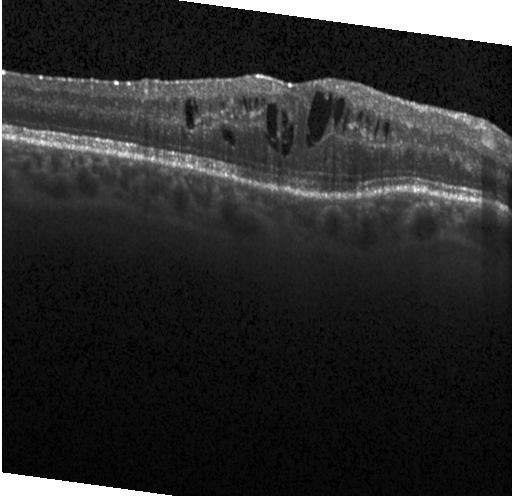
OCT B-scan. DME.